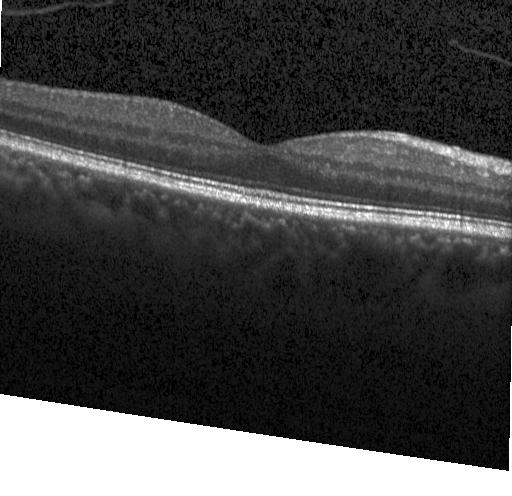

This B-scan demonstrates neither choroidal neovascularization, diabetic macular edema, nor drusen.